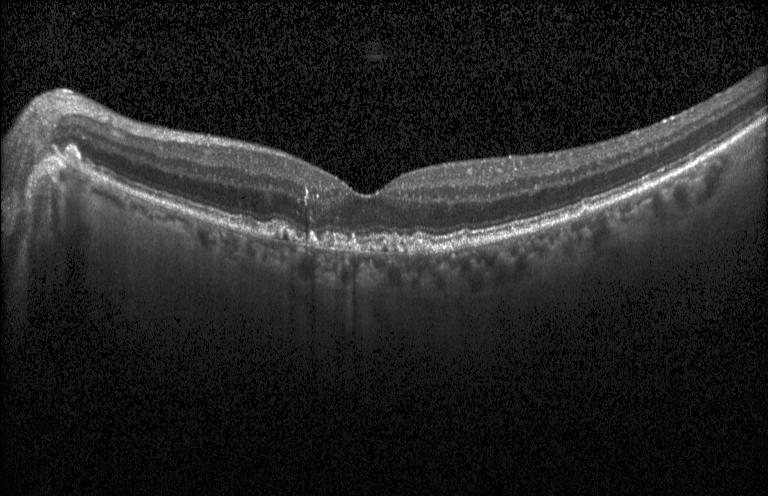
Acquired on a Heidelberg Spectralis. OCT line scan. Fovea-centered. Spectral-domain OCT — OCT finding: multiple drusen.